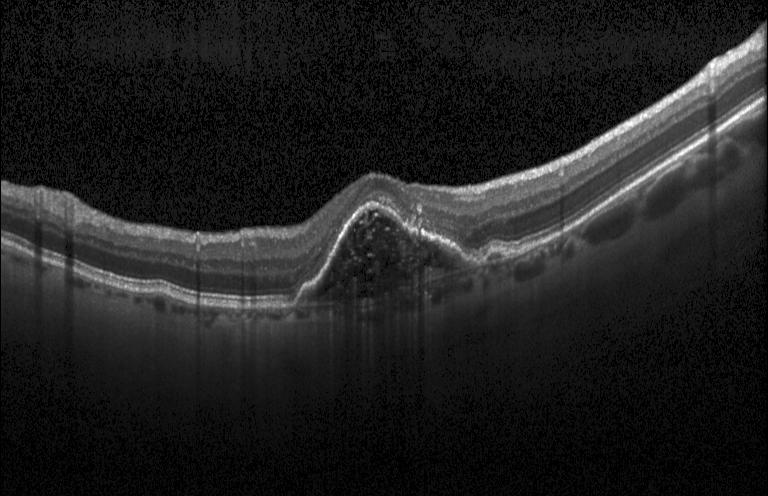

Horizontal scan through the fovea; spectral-domain OCT; OCT line scan. This B-scan demonstrates choroidal neovascularization (CNV).